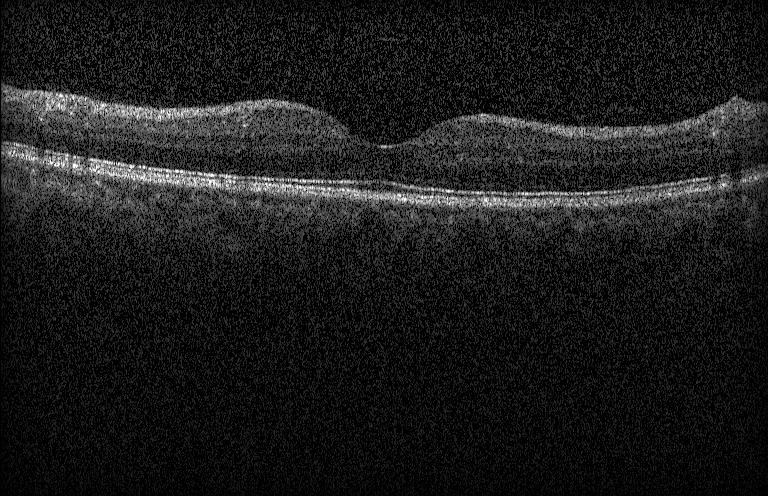

Macular OCT: no choroidal neovascularization, no diabetic macular edema, and no drusen.